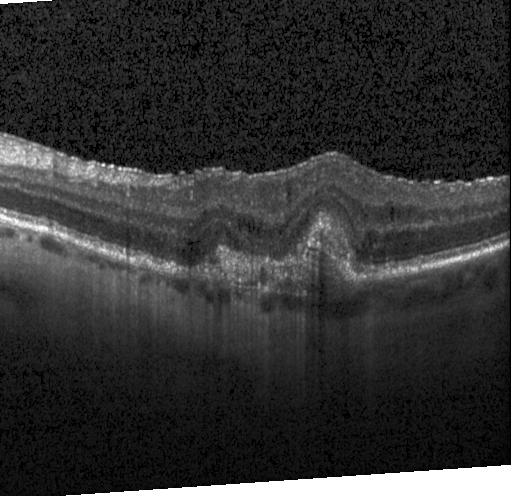
Retinal OCT B-scan; spectral-domain OCT; horizontal scan through the fovea. Impression: a choroidal neovascular membrane.